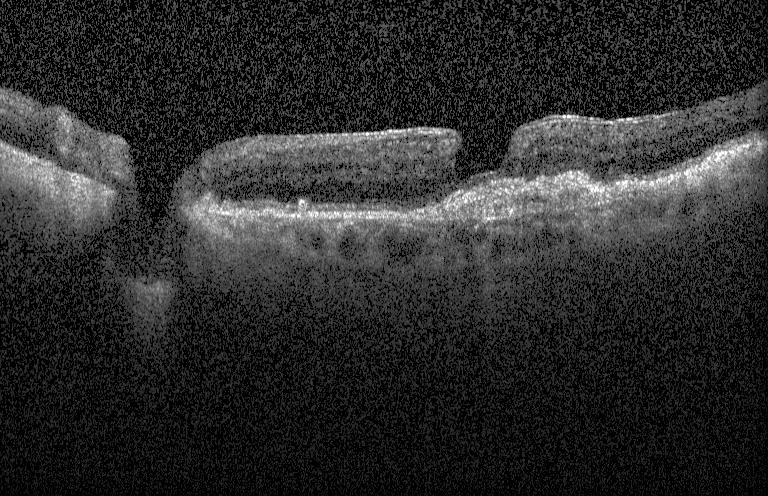
Finding: a choroidal neovascular membrane.